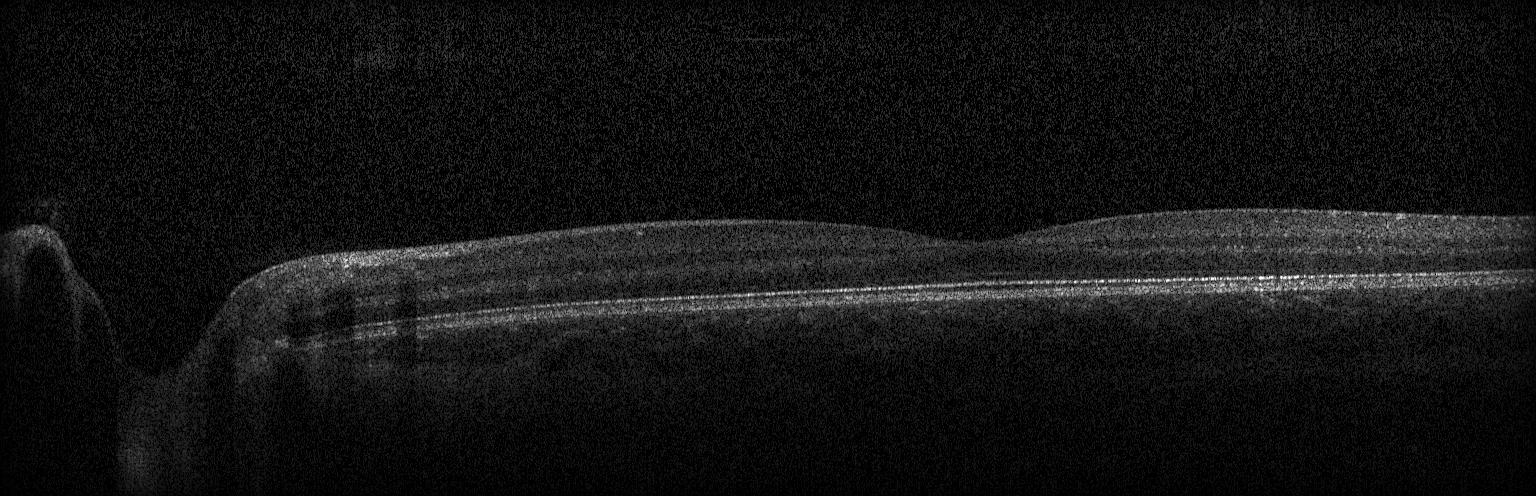

Finding: no choroidal neovascularization, no diabetic macular edema, and no drusen.